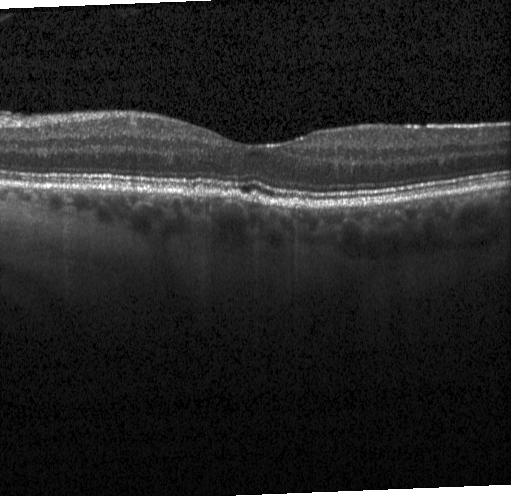

Impression: drusen.